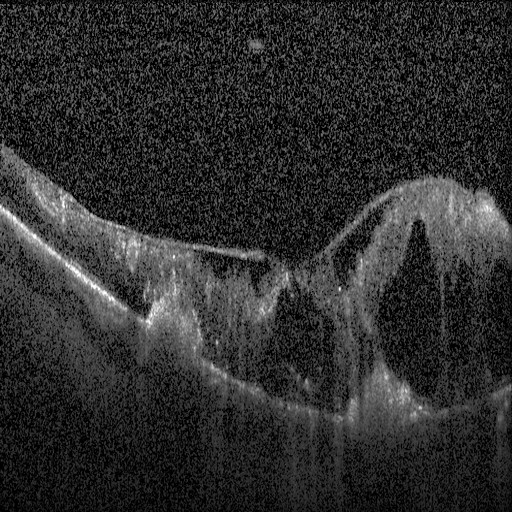

This B-scan demonstrates diabetic macular edema (DME).